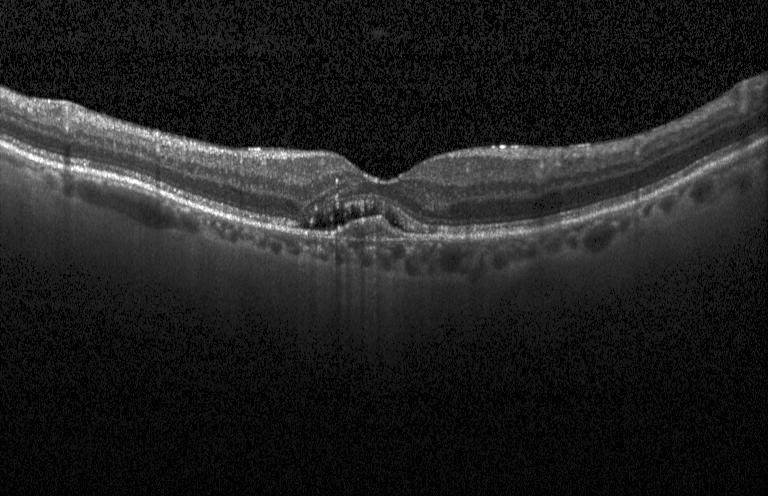
OCT finding: a choroidal neovascular membrane.